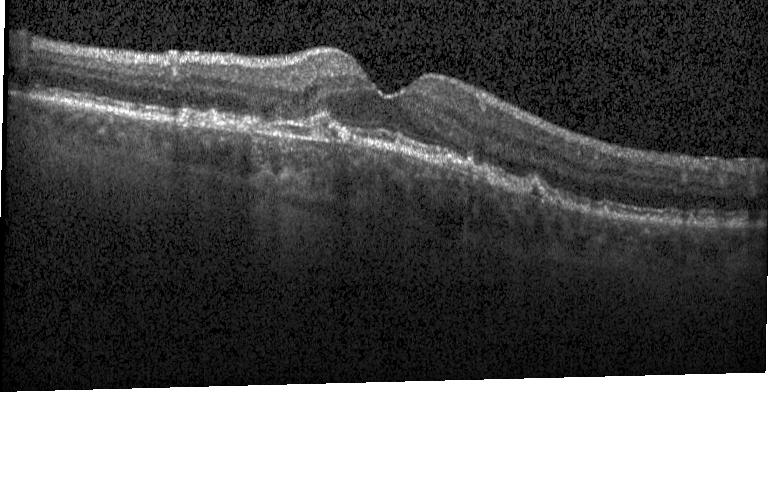
Assessment: a choroidal neovascular membrane.